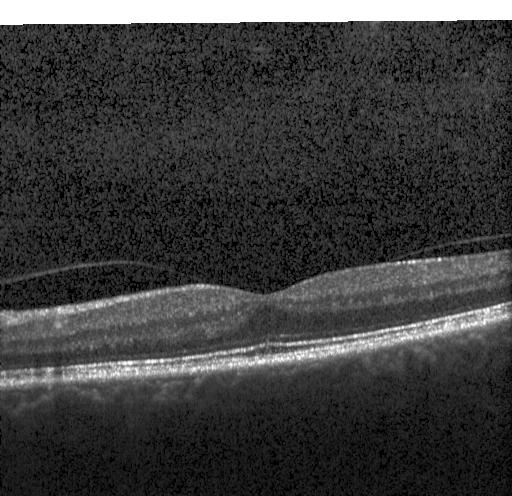

SD-OCT · retinal OCT B-scan · Heidelberg Spectralis · through the macula
Macular OCT: no evidence of choroidal neovascularization, diabetic macular edema, or drusen.